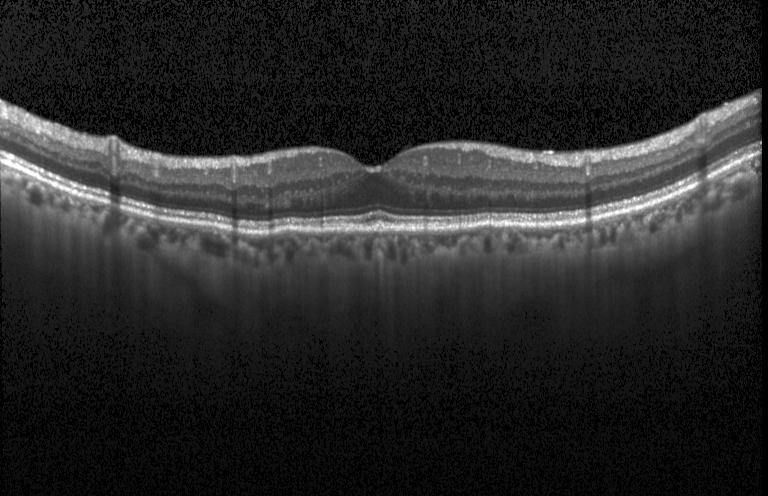
Acquired on a Heidelberg Spectralis; OCT line scan — Impression: no evidence of choroidal neovascularization, diabetic macular edema, or drusen.